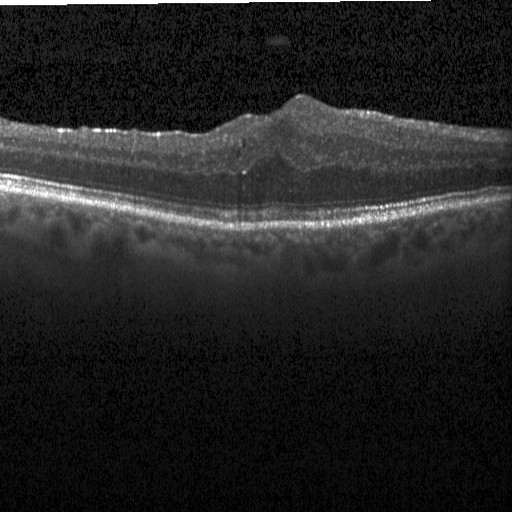 Through the macula · retinal OCT cross-section · spectral-domain OCT.
Assessment: diabetic macular edema.